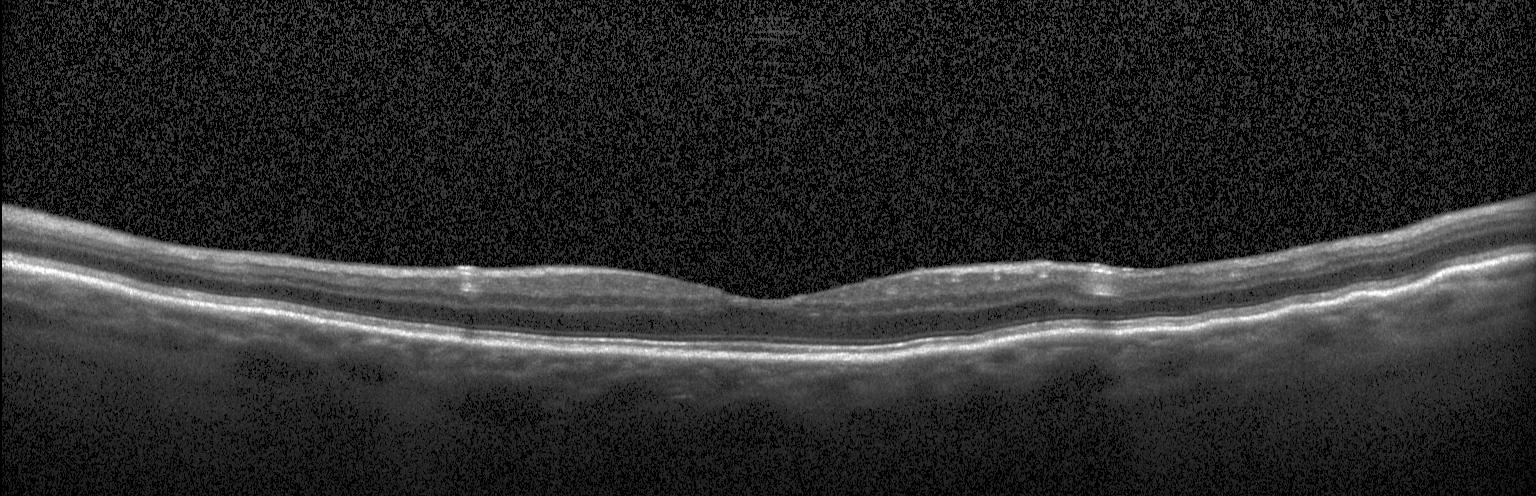 Finding: neither CNV, DME, nor drusen.